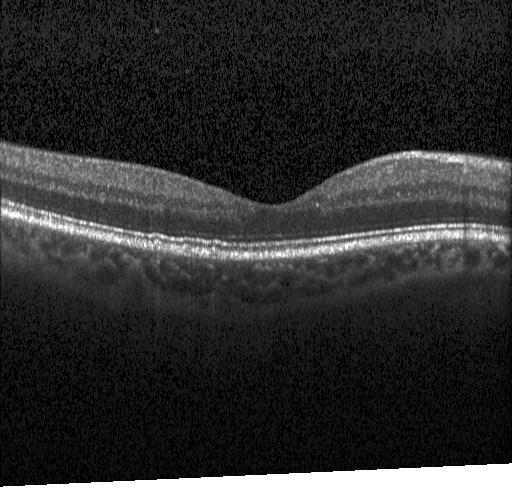 Impression: no choroidal neovascularization, no diabetic macular edema, and no drusen.